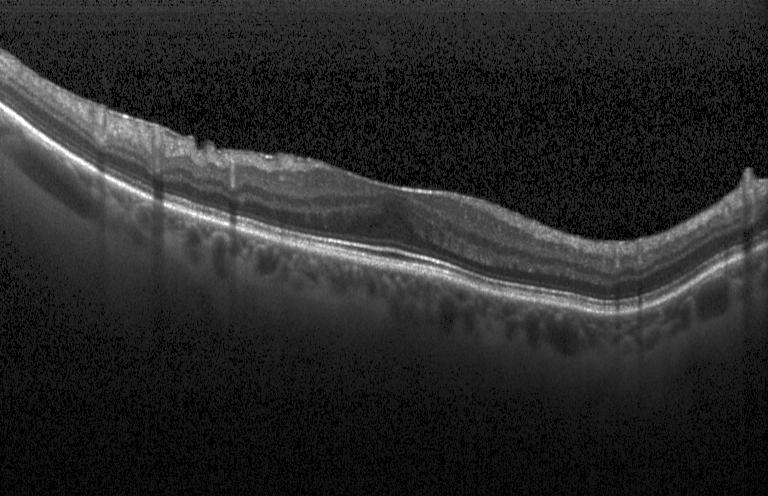

Acquired on a Heidelberg Spectralis; through the macula; retinal OCT cross-section. Finding: no choroidal neovascularization, diabetic macular edema, or drusen.